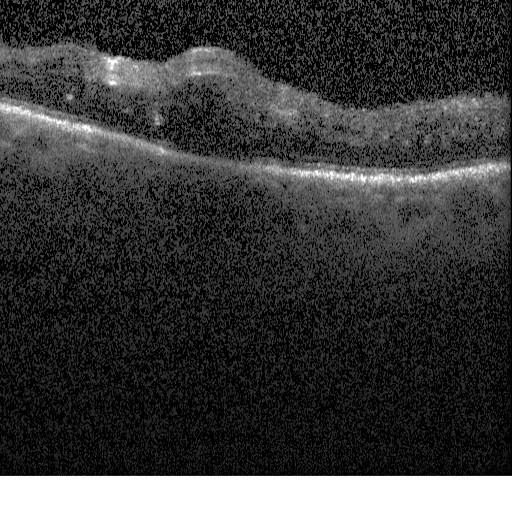

Fovea-centered. OCT line scan
Diagnosis: diabetic macular edema (DME).